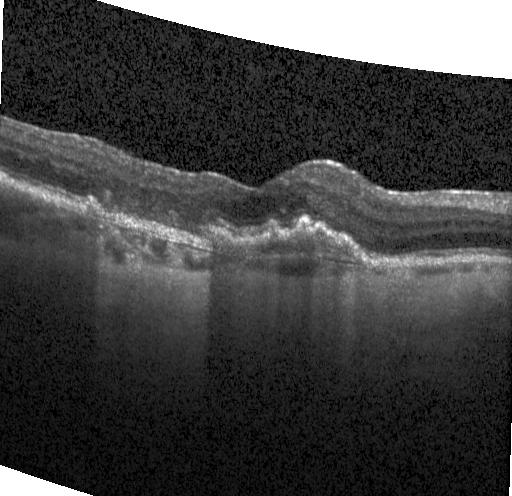
OCT B-scan. Finding: a choroidal neovascular membrane.